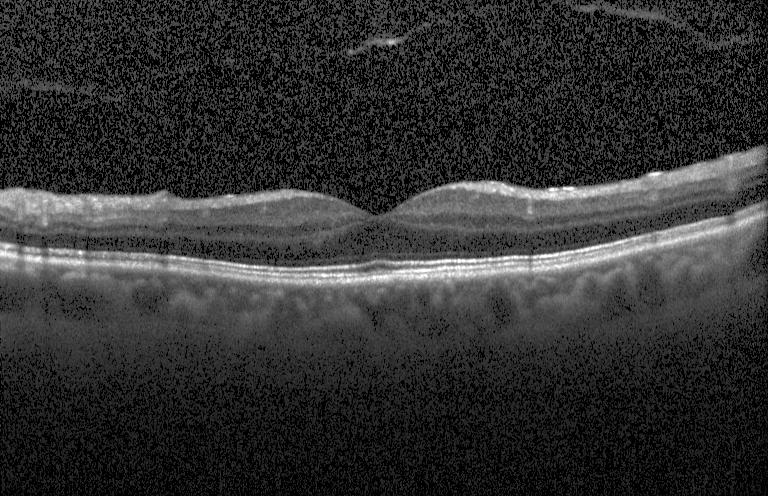
Dx: neither choroidal neovascularization, diabetic macular edema, nor drusen.